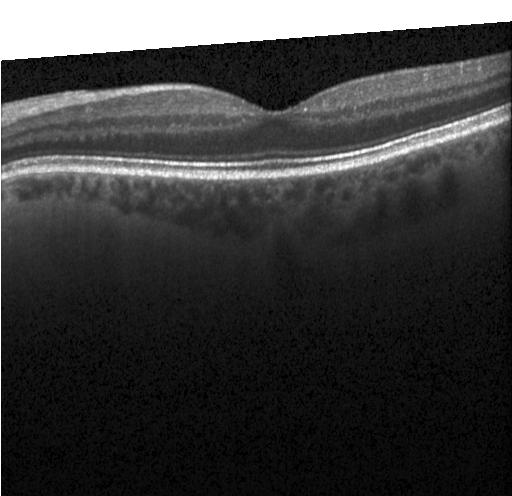

OCT B-scan — Diagnosis: neither CNV, DME, nor drusen.